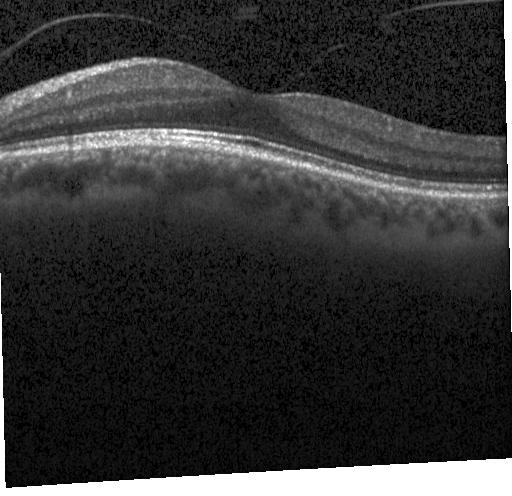 Fovea-centered; SD-OCT; Heidelberg Spectralis; optical coherence tomography scan
OCT finding: no CNV, DME, or drusen.